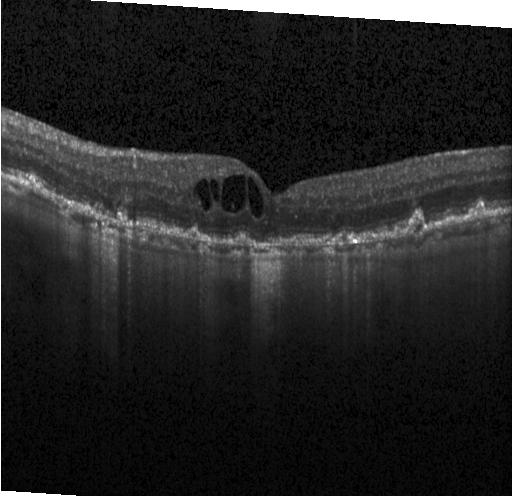
OCT line scan — Macular OCT: a choroidal neovascular membrane.